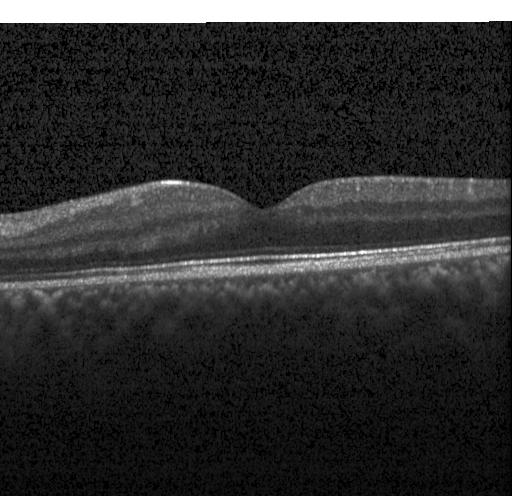

OCT finding: no choroidal neovascularization, diabetic macular edema, or drusen.